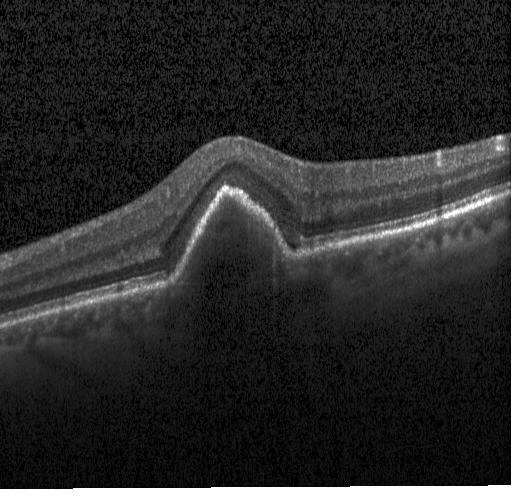

Spectral-domain OCT B-scan: a choroidal neovascular membrane.